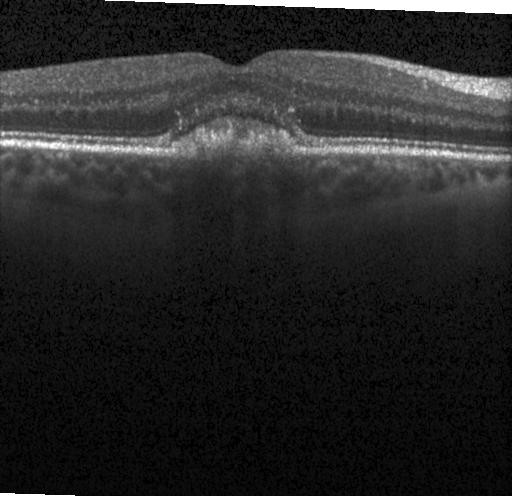
Spectral-domain optical coherence tomography, OCT B-scan, through the macula, acquired on a Heidelberg Spectralis.
Diagnosis: a choroidal neovascular membrane.